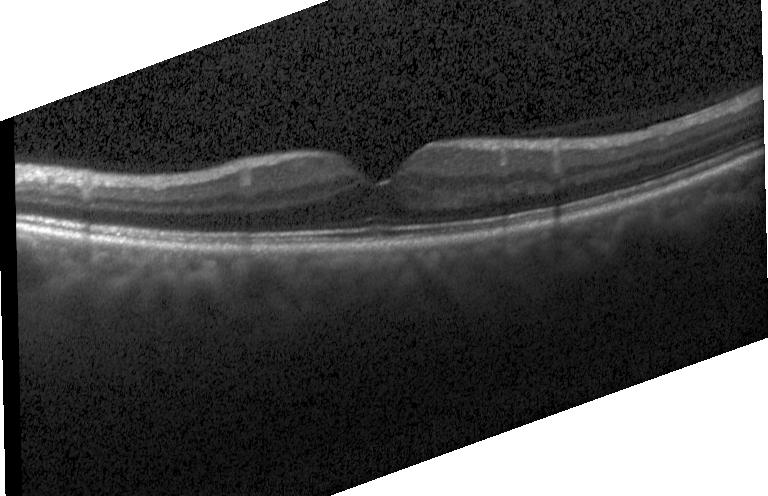
Impression: no choroidal neovascularization, no diabetic macular edema, and no drusen.